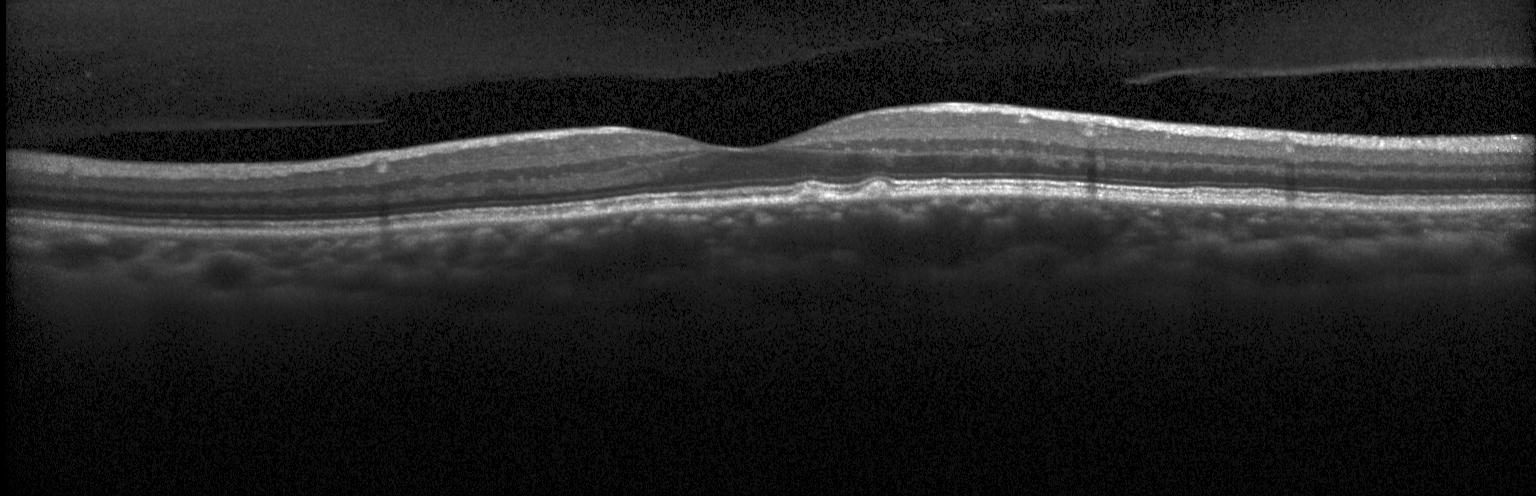 This B-scan demonstrates sub-RPE drusenoid deposits.